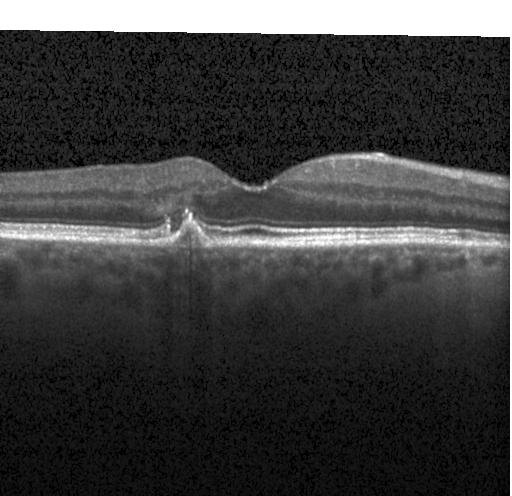

Macular OCT demonstrating sub-RPE drusenoid deposits.